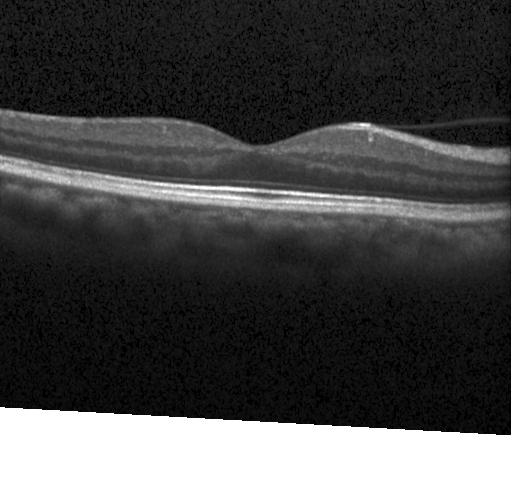

SD-OCT. Instrument: Heidelberg Spectralis. Macular scan. OCT line scan. Diagnosis: no evidence of choroidal neovascularization, diabetic macular edema, or drusen.